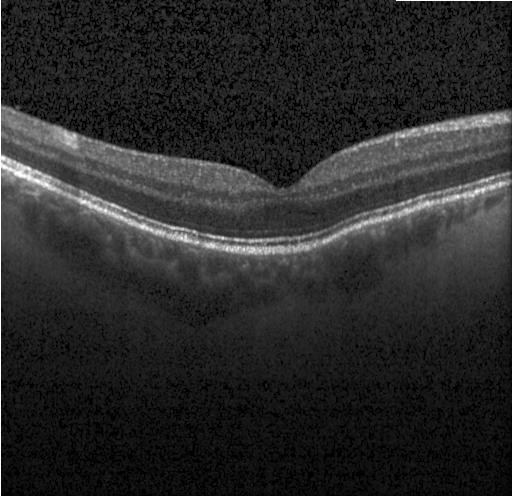
Through the macula, optical coherence tomography scan, spectral-domain OCT — The scan shows no choroidal neovascularization, diabetic macular edema, or drusen.